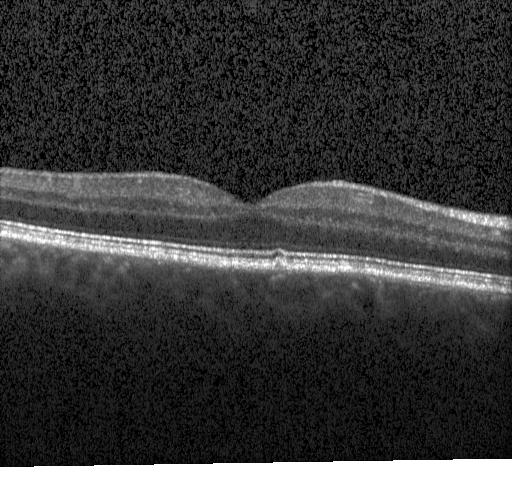
Finding: multiple drusen.